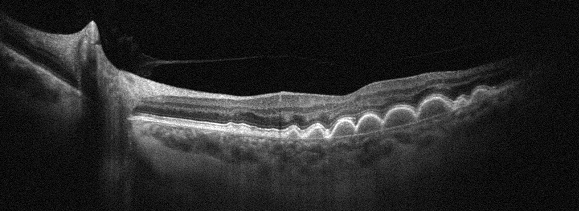

Diagnosis: age-related macular degeneration (AMD).